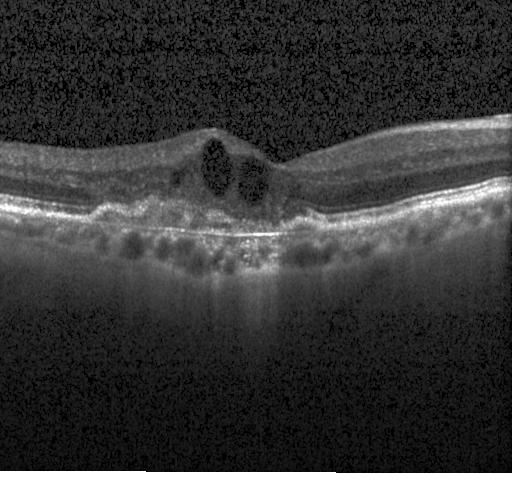
Heidelberg Spectralis OCT system, optical coherence tomography B-scan
This B-scan demonstrates a choroidal neovascular membrane.